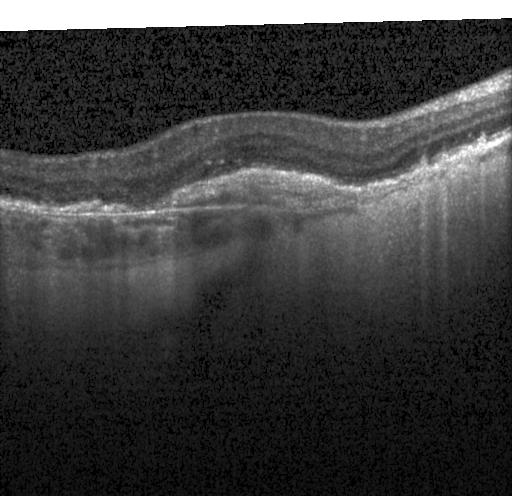
Assessment: CNV.